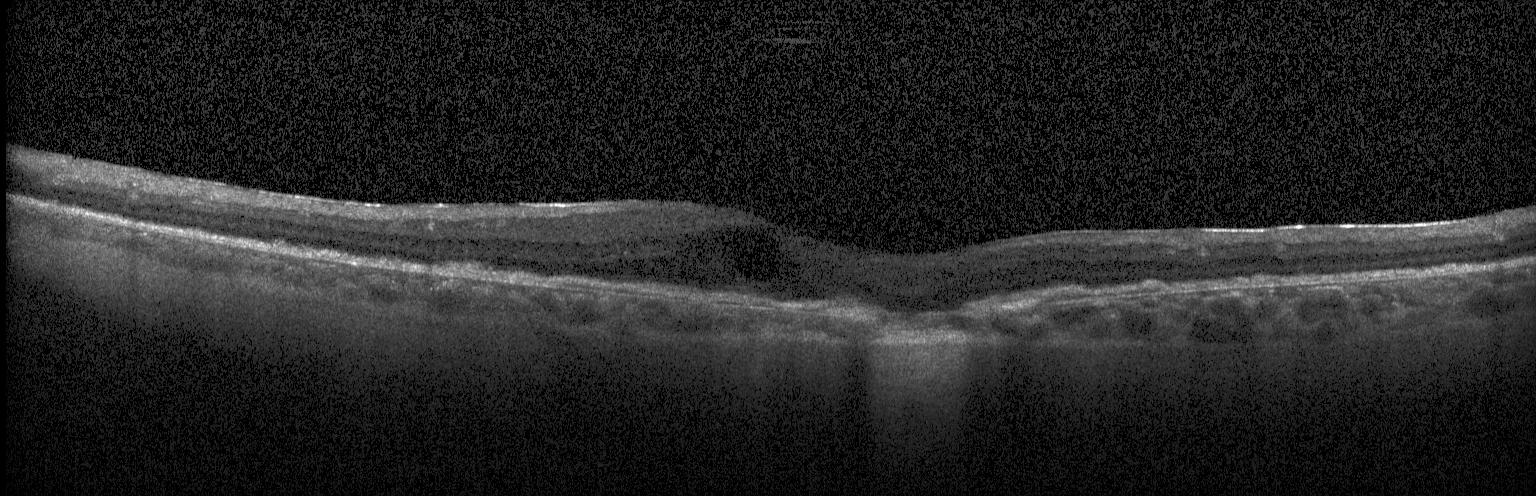

OCT line scan
A choroidal neovascular membrane.